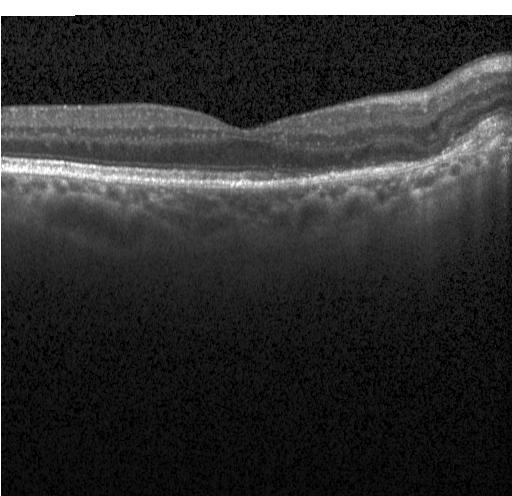 Impression: choroidal neovascularization (CNV).